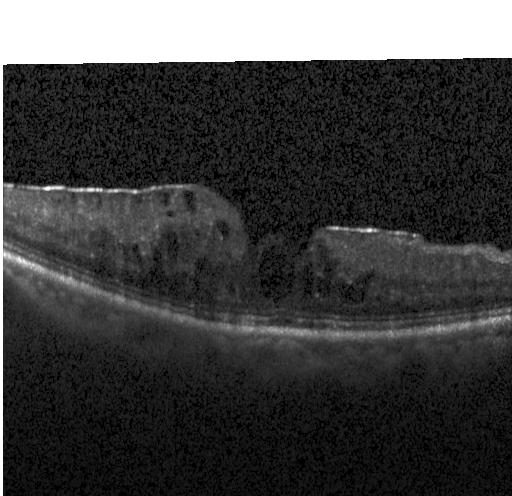 Assessment: DME.